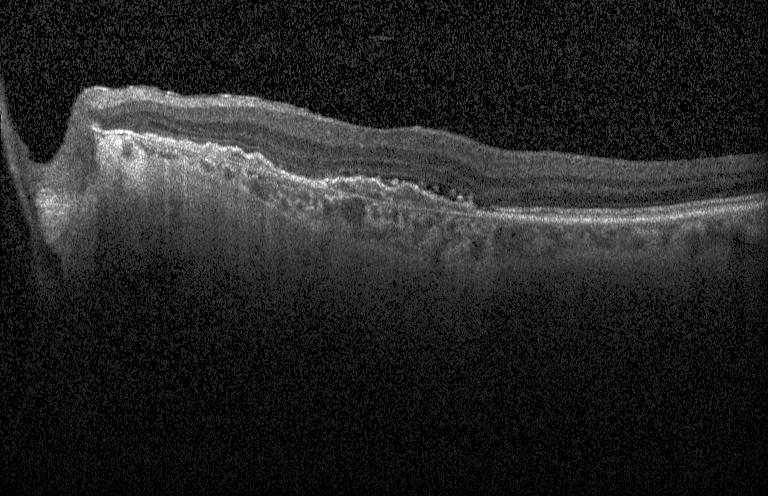
Acquired on a Heidelberg Spectralis; optical coherence tomography B-scan. Impression: a choroidal neovascular membrane.